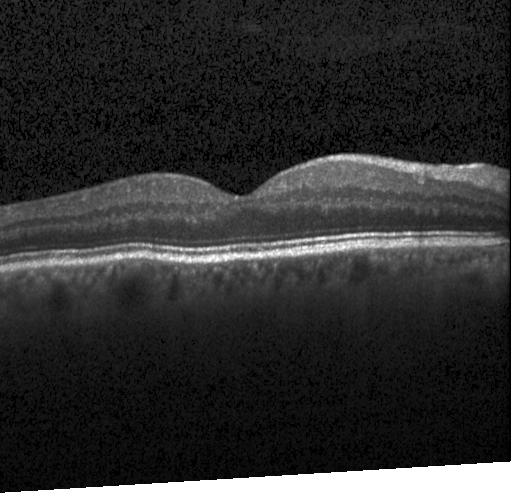 Centered on the fovea, optical coherence tomography B-scan — Macular OCT: no CNV, no DME, and no drusen.